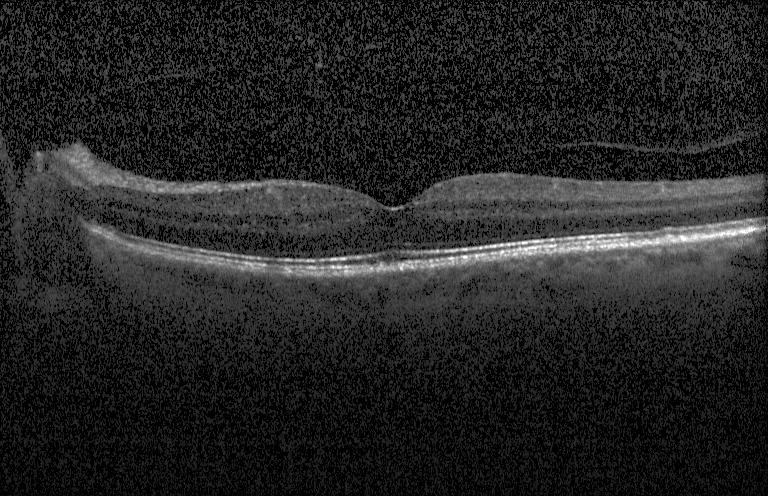

OCT scan showing no choroidal neovascularization, diabetic macular edema, or drusen.